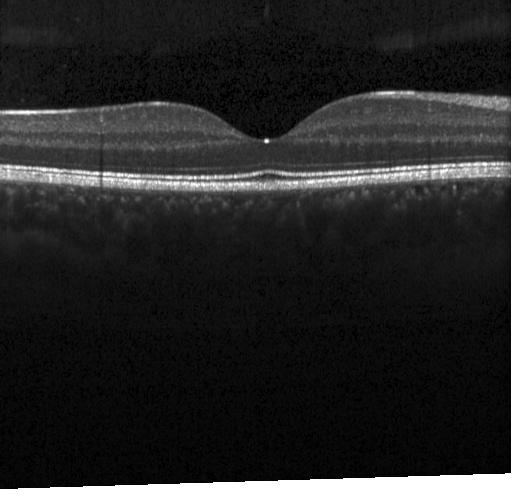
Fovea-centered, spectral-domain OCT, retinal OCT cross-section, Heidelberg Spectralis OCT system.
Diagnosis: no evidence of choroidal neovascularization, diabetic macular edema, or drusen.